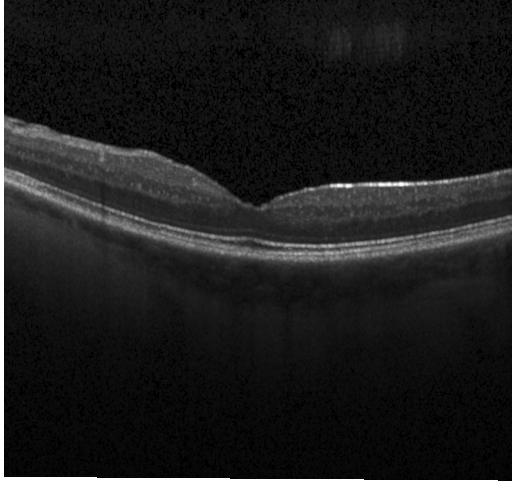 Retinal OCT cross-section. Assessment: no evidence of CNV, DME, or drusen.